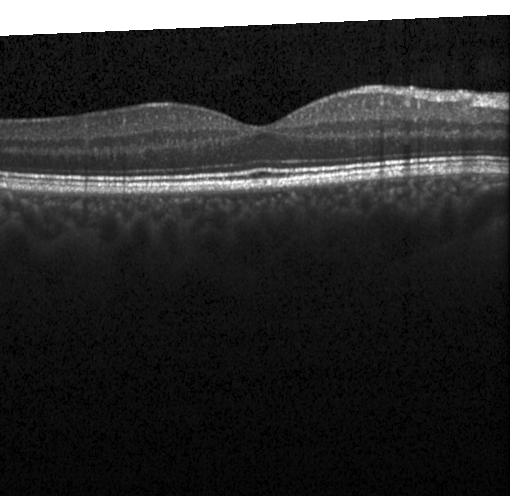

Macular OCT demonstrating no choroidal neovascularization, no diabetic macular edema, and no drusen.